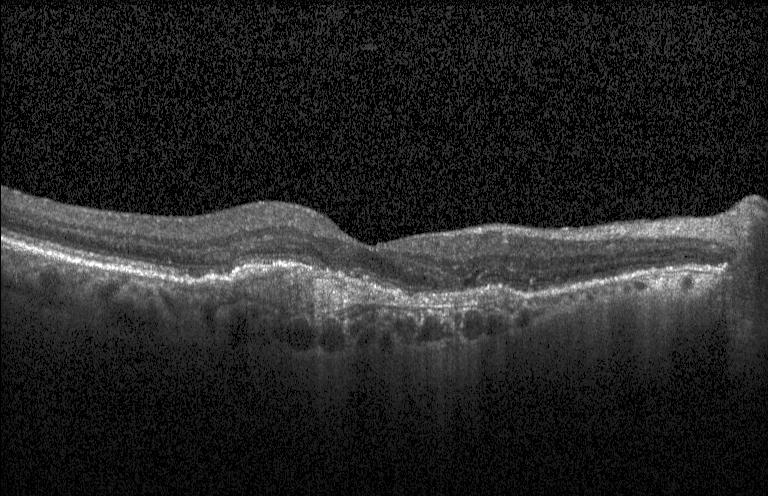
OCT B-scan showing choroidal neovascularization (CNV).